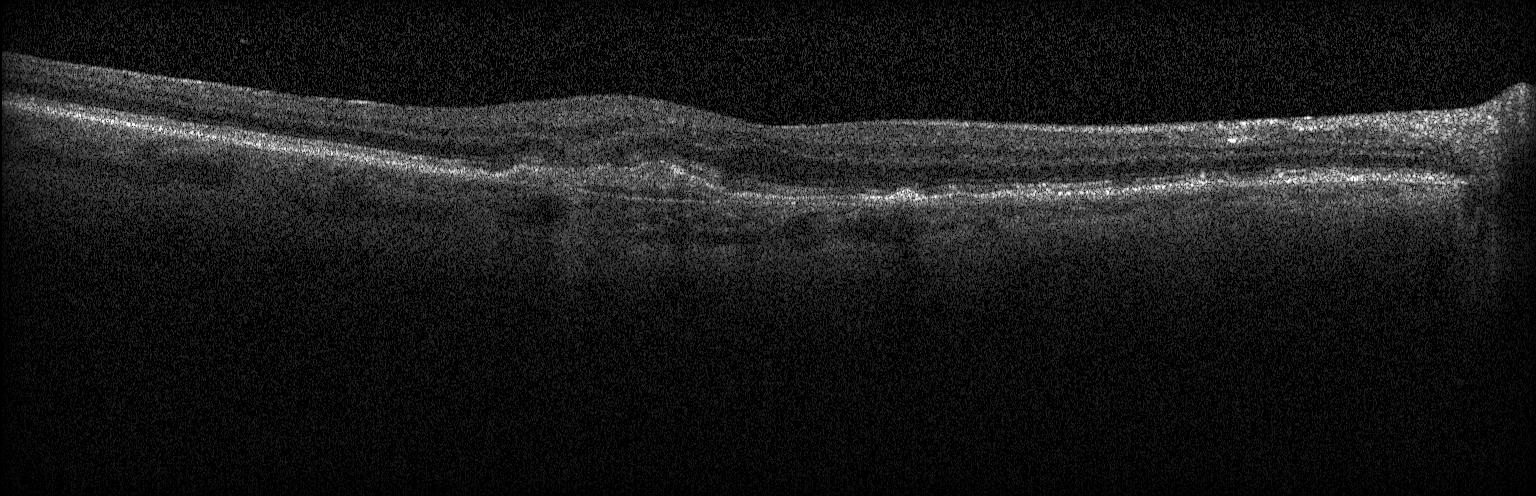 Spectral-domain OCT B-scan: choroidal neovascularization (CNV).